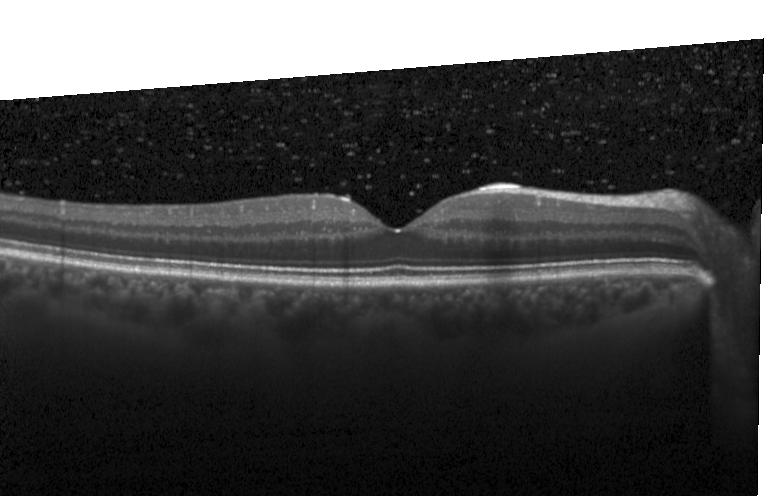 Macular OCT demonstrating no CNV, no DME, and no drusen.